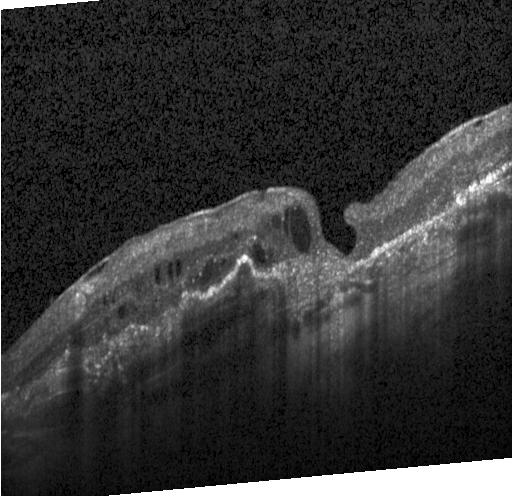
OCT line scan — Finding: choroidal neovascularization (CNV).